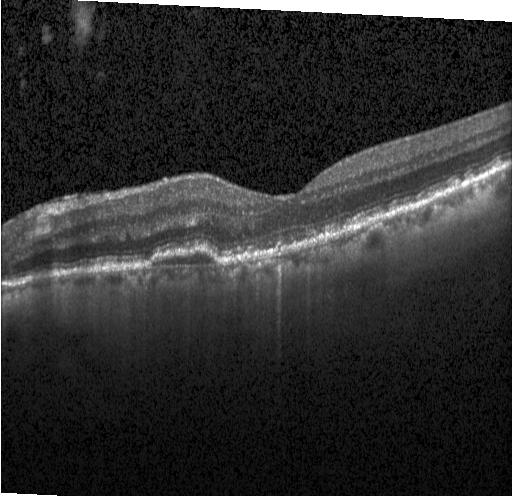

OCT finding: choroidal neovascularization.